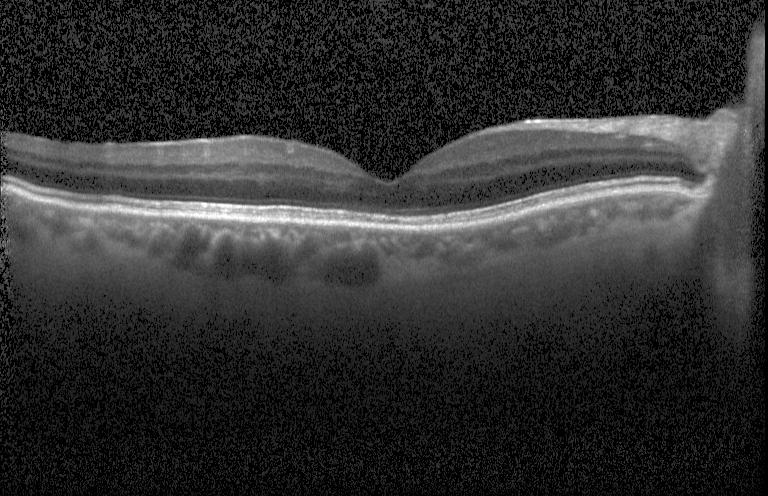 Spectral-domain OCT B-scan: neither choroidal neovascularization, diabetic macular edema, nor drusen.